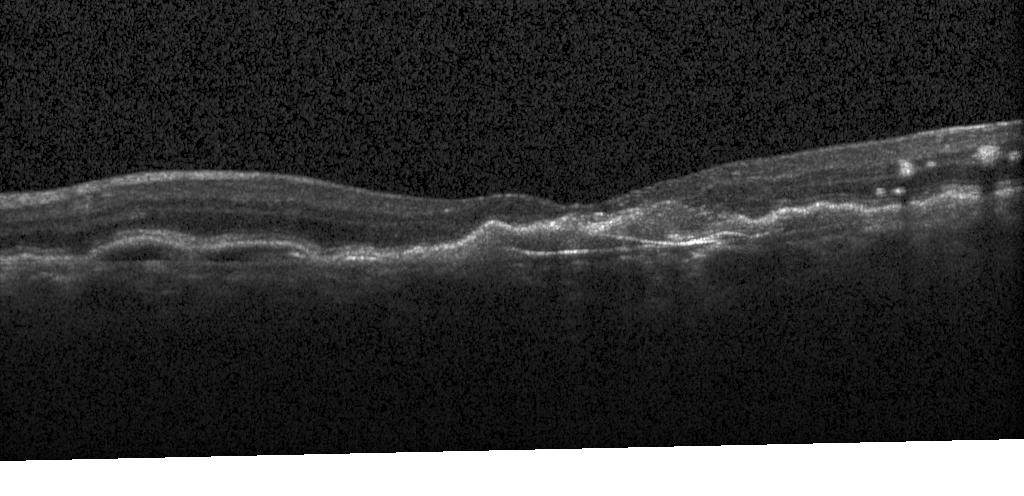

SD-OCT · OCT line scan · fovea-centered.
This B-scan demonstrates a choroidal neovascular membrane.